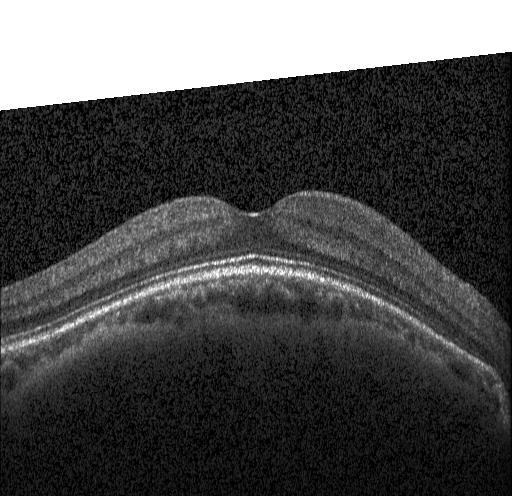

Fovea-centered; Heidelberg Spectralis OCT system; spectral-domain OCT; optical coherence tomography scan
Impression: no CNV, DME, or drusen.